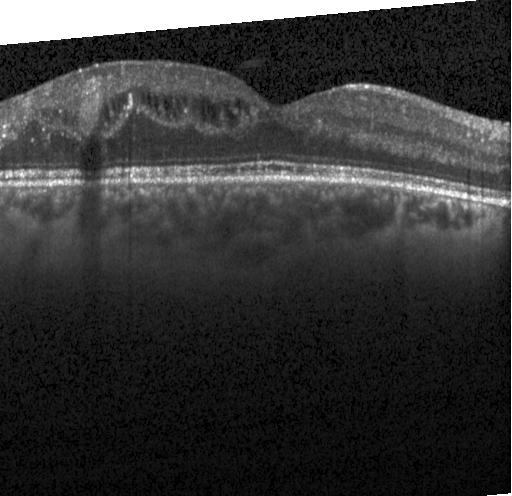 Finding: diabetic macular edema.